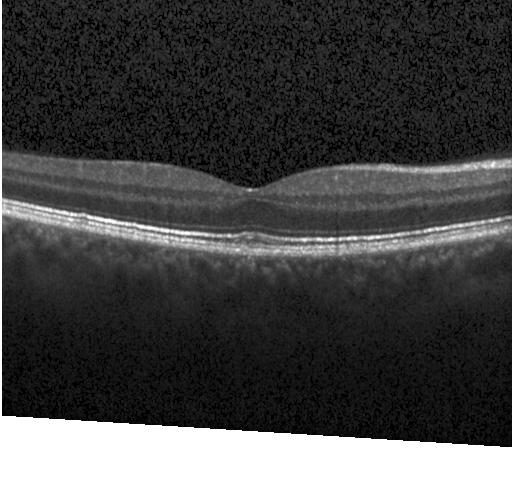

Macular OCT: neither choroidal neovascularization, diabetic macular edema, nor drusen.